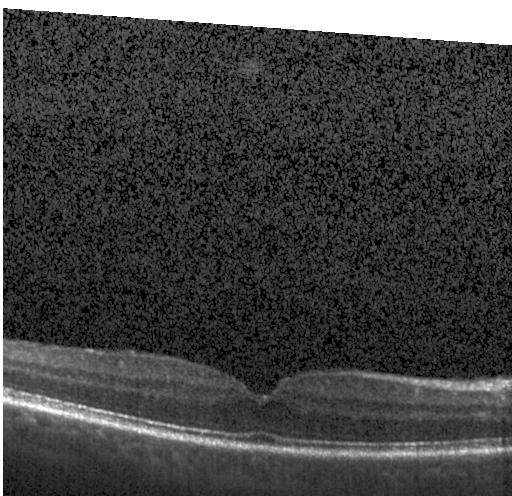

Horizontal scan through the fovea. Retinal OCT B-scan. SD-OCT. Macular OCT: no evidence of CNV, DME, or drusen.